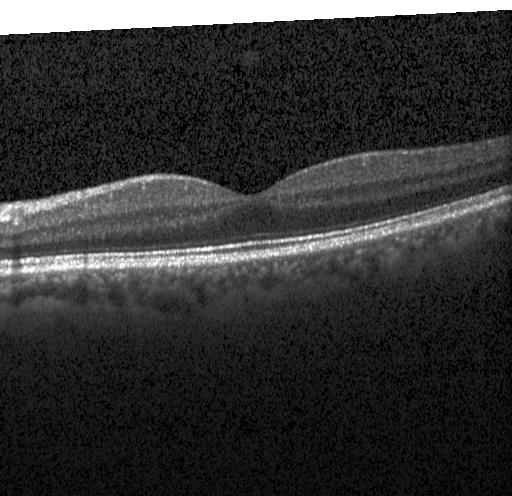 Retinal OCT cross-section. SD-OCT. Centered on the fovea. Heidelberg Spectralis.
The scan shows no evidence of choroidal neovascularization, diabetic macular edema, or drusen.